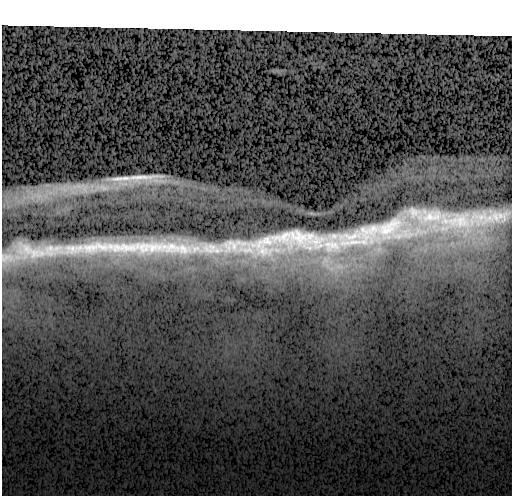 Spectral-domain optical coherence tomography. Instrument: Heidelberg Spectralis. Fovea-centered. OCT line scan — Finding: CNV.